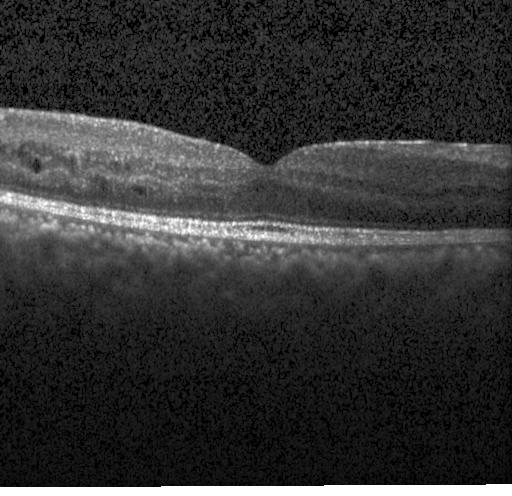
OCT B-scan showing diabetic macular edema.